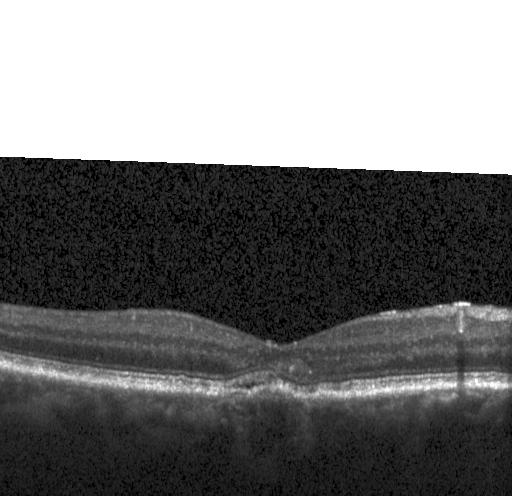 Dx: a choroidal neovascular membrane.